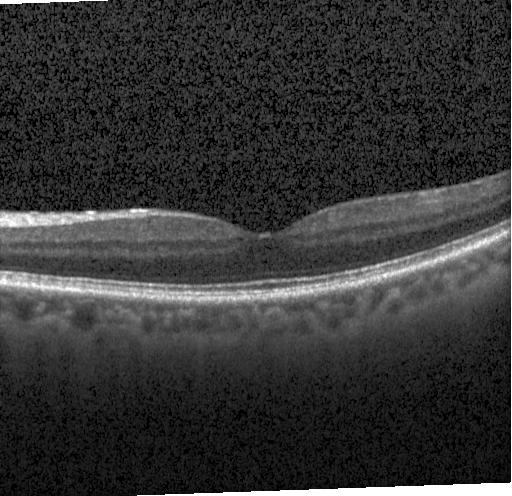

Centered on the fovea, OCT B-scan, Heidelberg Spectralis, spectral-domain OCT — Assessment: no evidence of choroidal neovascularization, diabetic macular edema, or drusen.